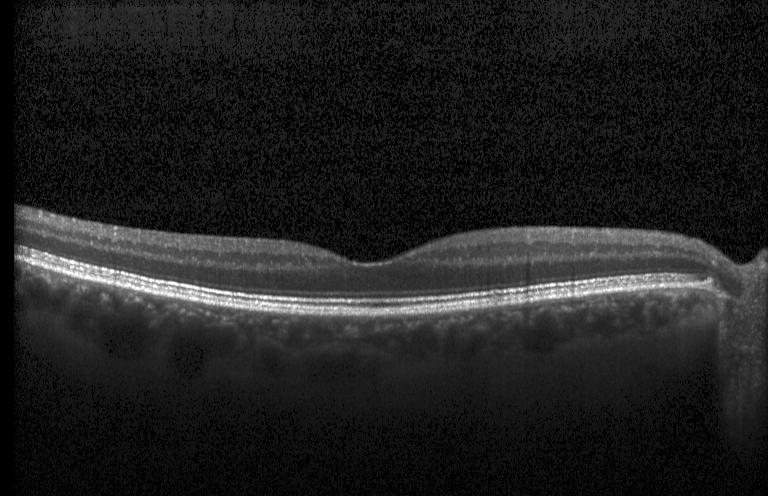

Optical coherence tomography scan. Heidelberg Spectralis OCT system. Spectral-domain optical coherence tomography
Diagnosis: no choroidal neovascularization, diabetic macular edema, or drusen.